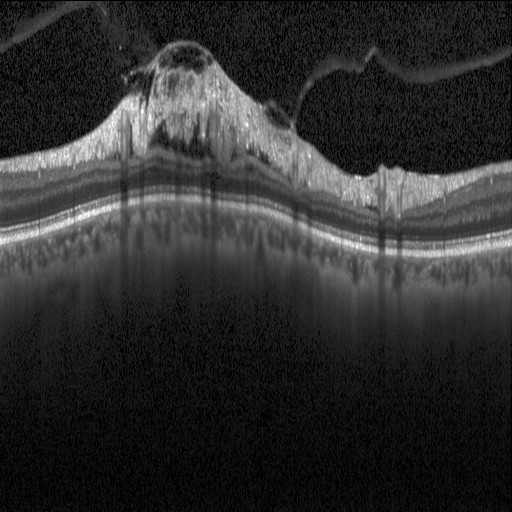

Finding: DME.